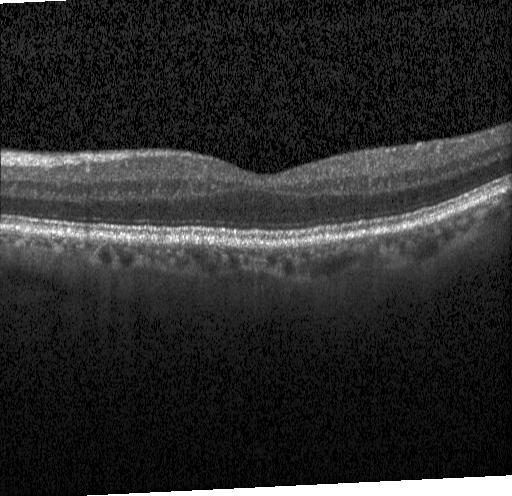

Diagnosis: no choroidal neovascularization, diabetic macular edema, or drusen.